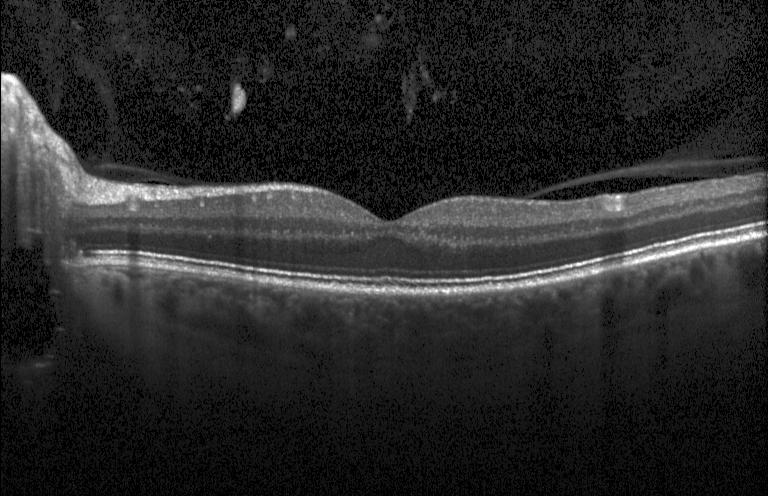
Acquired on a Heidelberg Spectralis; spectral-domain OCT; fovea-centered; optical coherence tomography B-scan. Impression: no choroidal neovascularization, no diabetic macular edema, and no drusen.